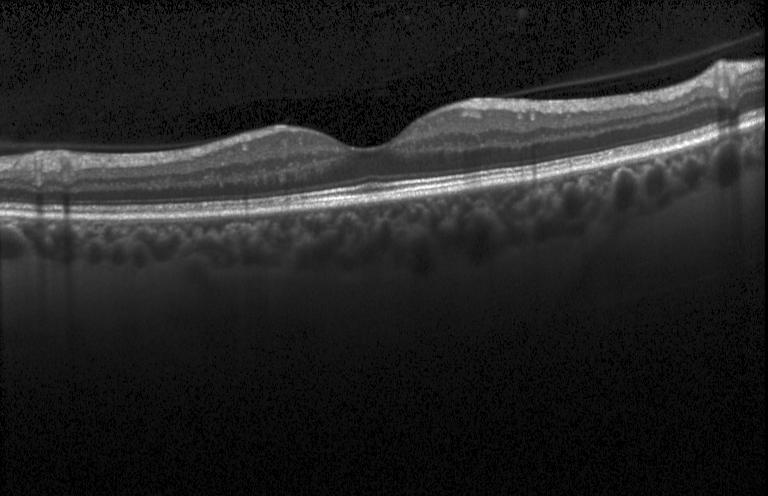 Heidelberg Spectralis, OCT line scan. Impression: neither choroidal neovascularization, diabetic macular edema, nor drusen.